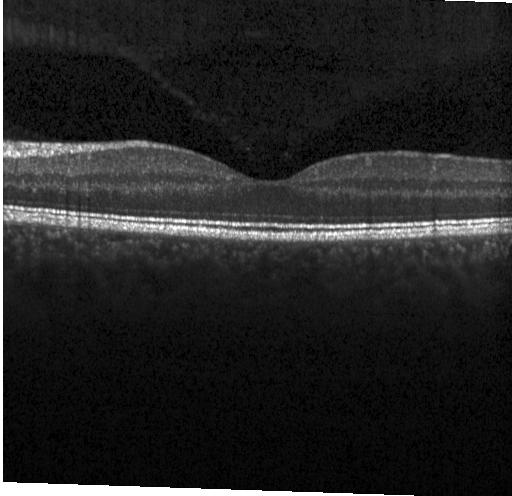 Finding: no choroidal neovascularization, no diabetic macular edema, and no drusen.